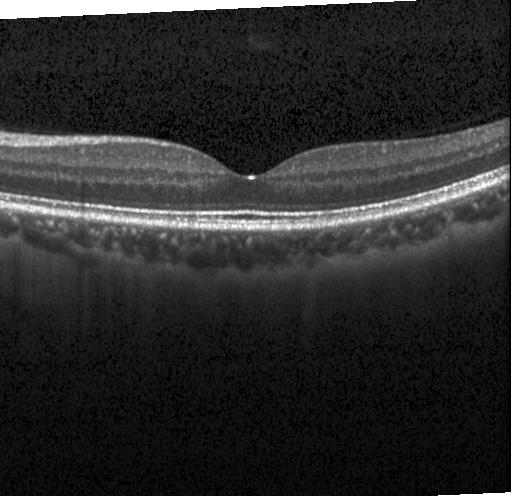
Macular OCT: neither choroidal neovascularization, diabetic macular edema, nor drusen.